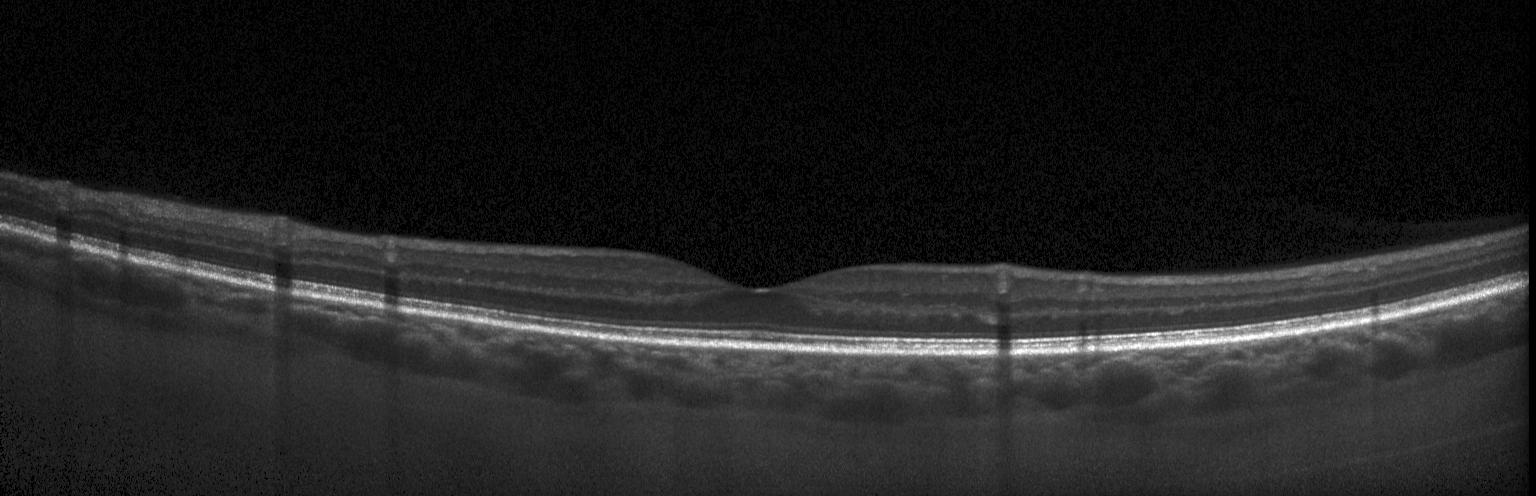
Retinal OCT B-scan, centered on the fovea, acquired on a Heidelberg Spectralis, spectral-domain OCT — OCT finding: neither CNV, DME, nor drusen.